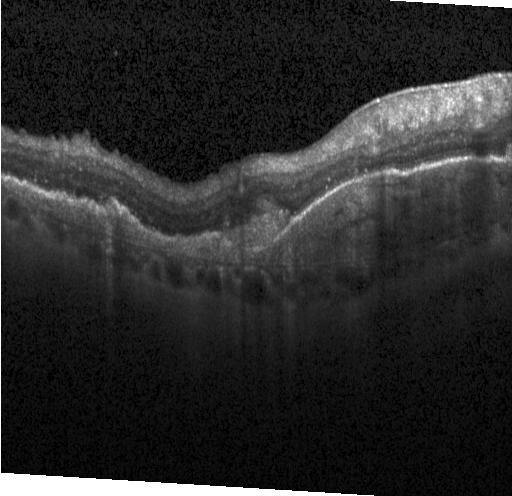 Macular scan, retinal OCT B-scan
Dx: a choroidal neovascular membrane.